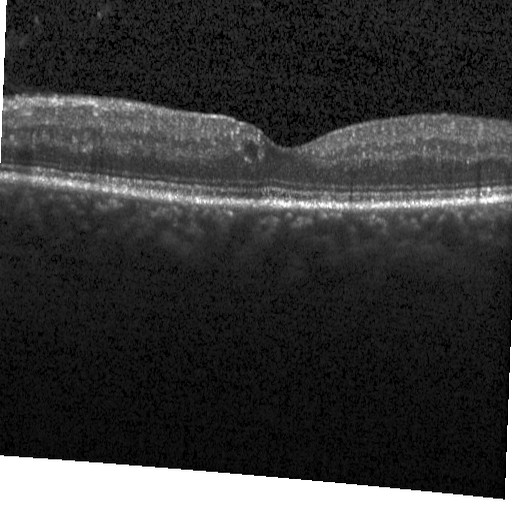 OCT line scan. Macular scan. Acquired on a Heidelberg Spectralis. Spectral-domain OCT. This B-scan demonstrates diabetic macular edema.